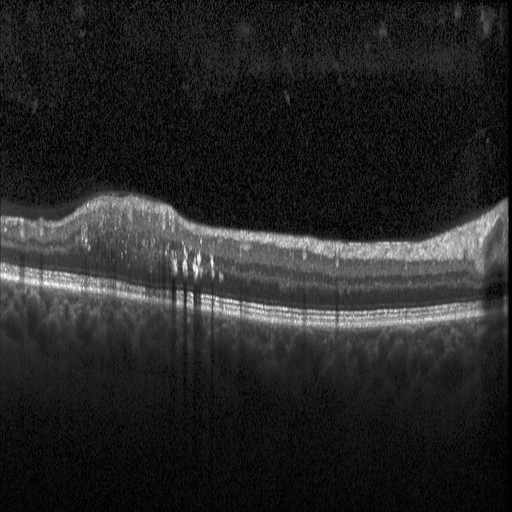 Heidelberg Spectralis · optical coherence tomography B-scan · spectral-domain optical coherence tomography
Macular OCT: diabetic macular edema.